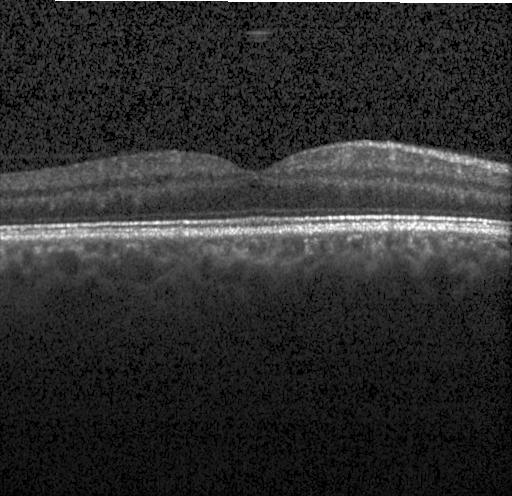 Retinal OCT cross-section · macular scan · acquired on a Heidelberg Spectralis · spectral-domain OCT. No evidence of choroidal neovascularization, diabetic macular edema, or drusen.